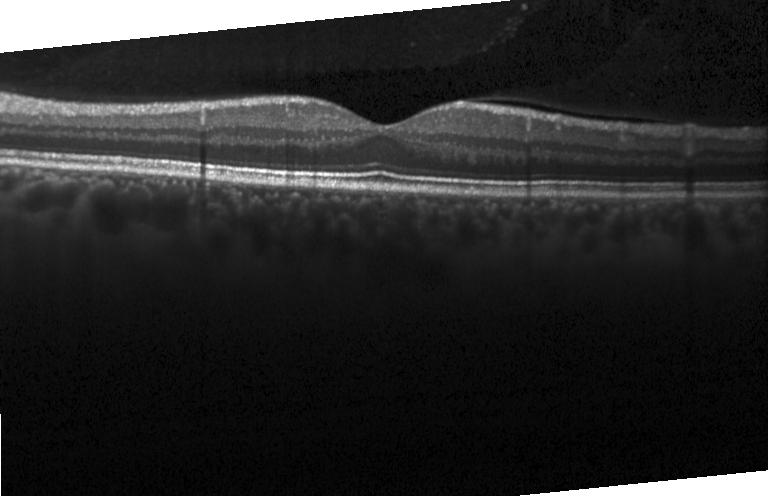 Impression: neither choroidal neovascularization, diabetic macular edema, nor drusen.